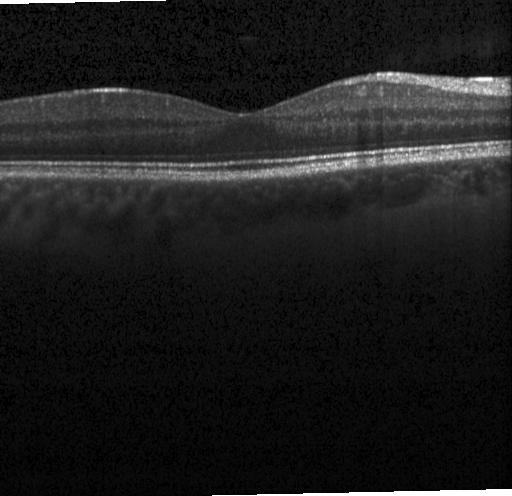
Retinal OCT cross-section — Diagnosis: neither choroidal neovascularization, diabetic macular edema, nor drusen.